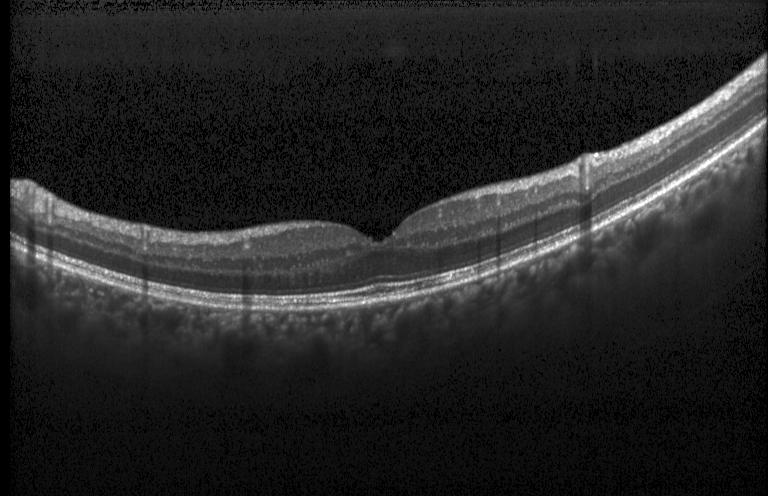

Horizontal scan through the fovea; optical coherence tomography B-scan — Macular OCT: neither choroidal neovascularization, diabetic macular edema, nor drusen.